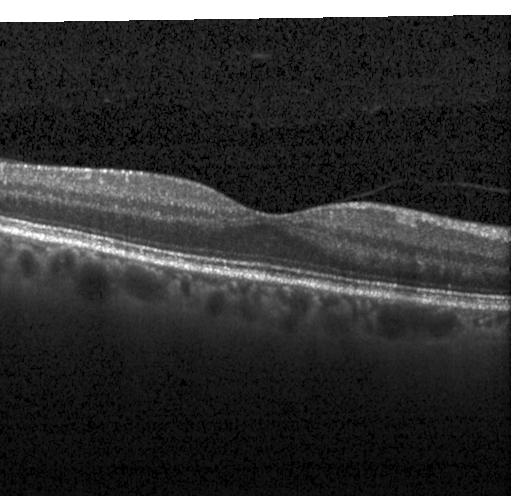
Retinal OCT B-scan.
Impression: no choroidal neovascularization, no diabetic macular edema, and no drusen.